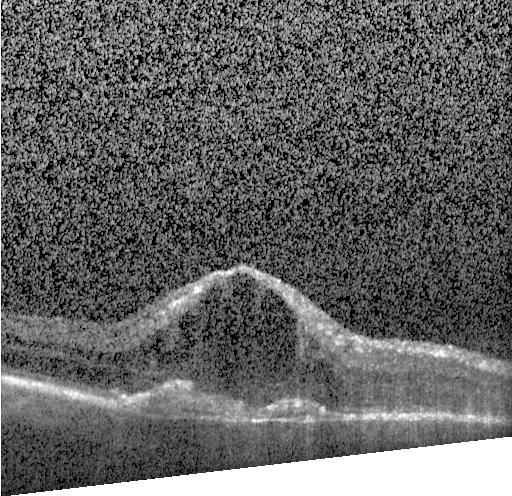 OCT B-scan. SD-OCT. Macular OCT: a choroidal neovascular membrane.